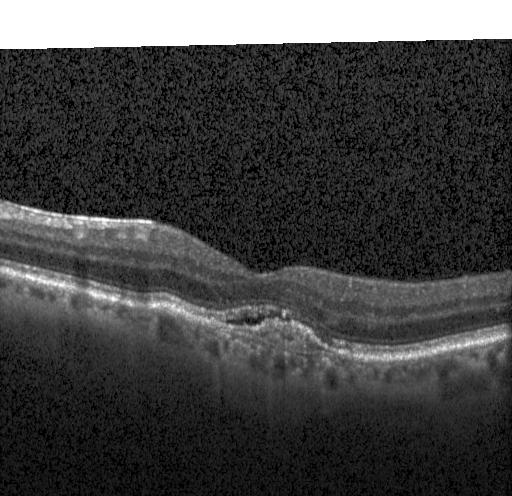

Finding: a choroidal neovascular membrane.